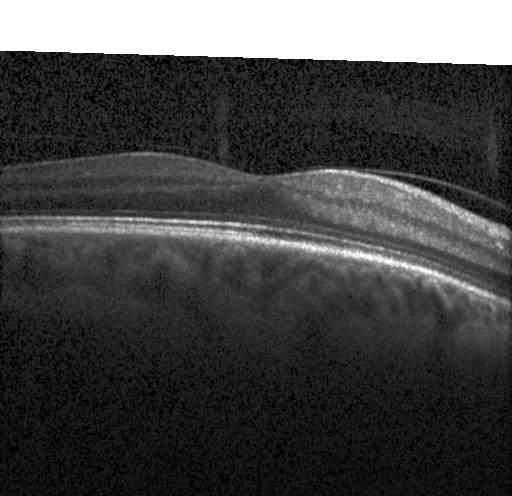
Retinal OCT cross-section showing no choroidal neovascularization, no diabetic macular edema, and no drusen.